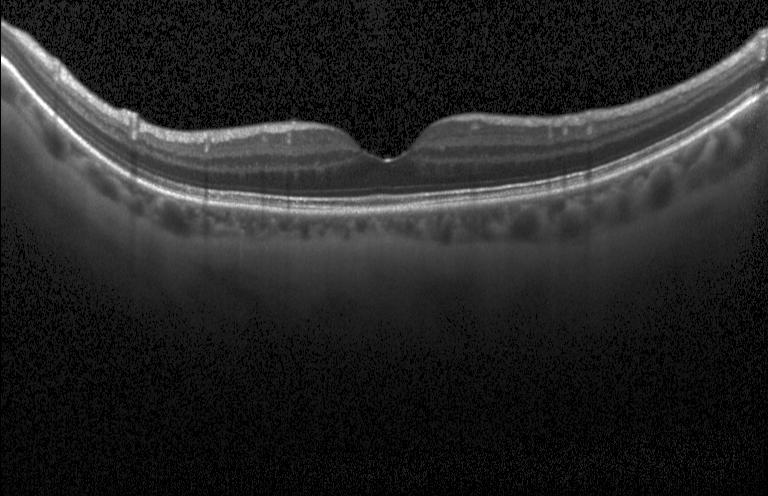
OCT line scan. Instrument: Heidelberg Spectralis — Impression: no choroidal neovascularization, diabetic macular edema, or drusen.